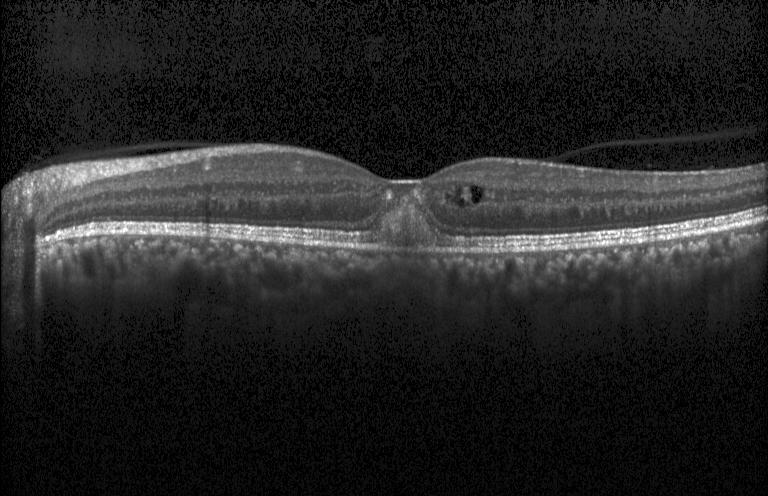
A choroidal neovascular membrane.